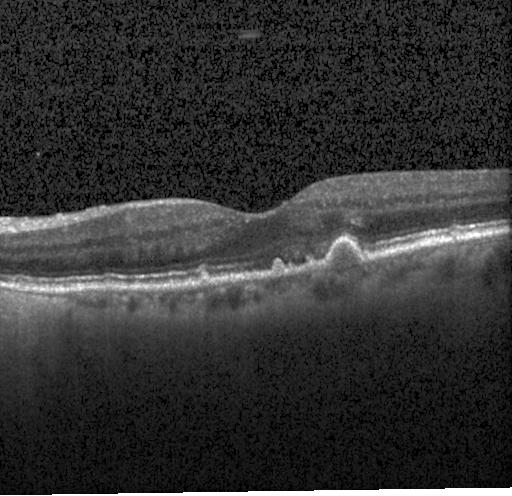
Macular OCT: multiple drusen.